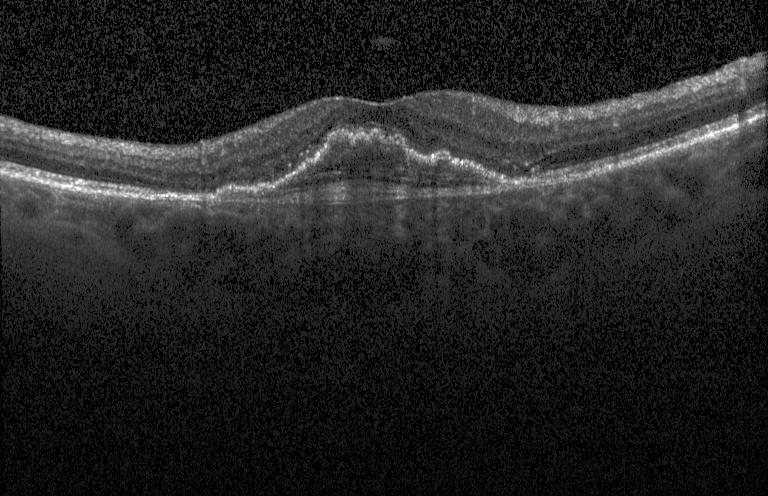

Fovea-centered, retinal OCT B-scan
Diagnosis: a choroidal neovascular membrane.